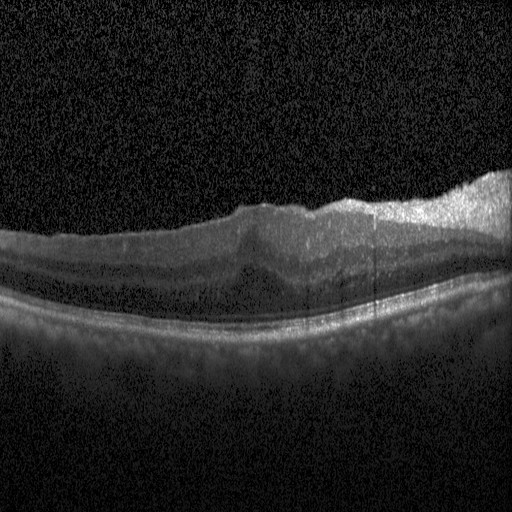
Heidelberg Spectralis OCT system · fovea-centered · OCT B-scan — Macular OCT: diabetic macular edema.